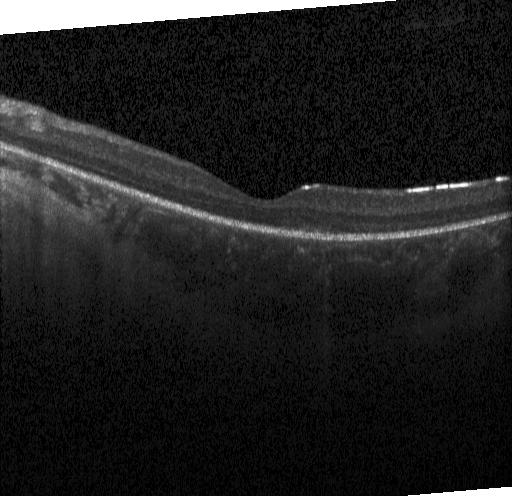
OCT line scan — Diagnosis: neither choroidal neovascularization, diabetic macular edema, nor drusen.